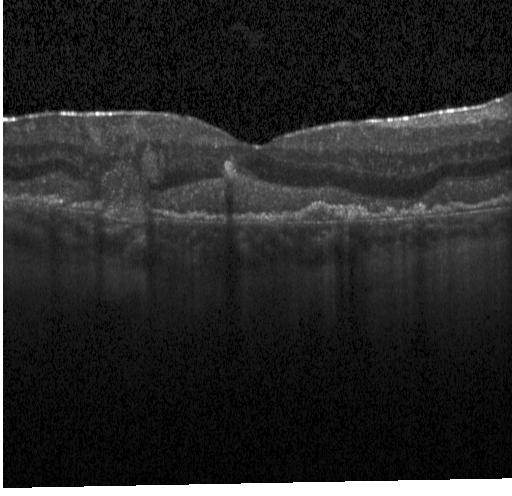
OCT line scan · spectral-domain optical coherence tomography · fovea-centered · acquired on a Heidelberg Spectralis — Dx: CNV.